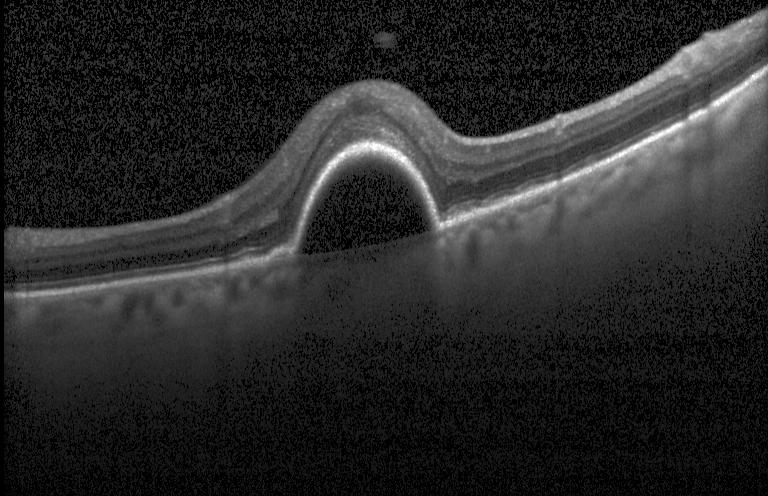

Macular OCT: choroidal neovascularization (CNV).